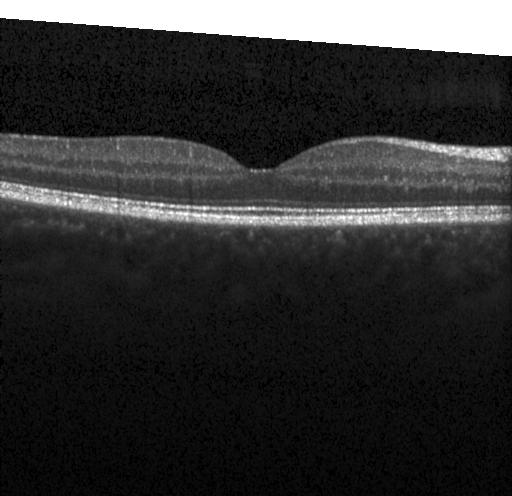

Retinal OCT cross-section.
This B-scan demonstrates no evidence of choroidal neovascularization, diabetic macular edema, or drusen.